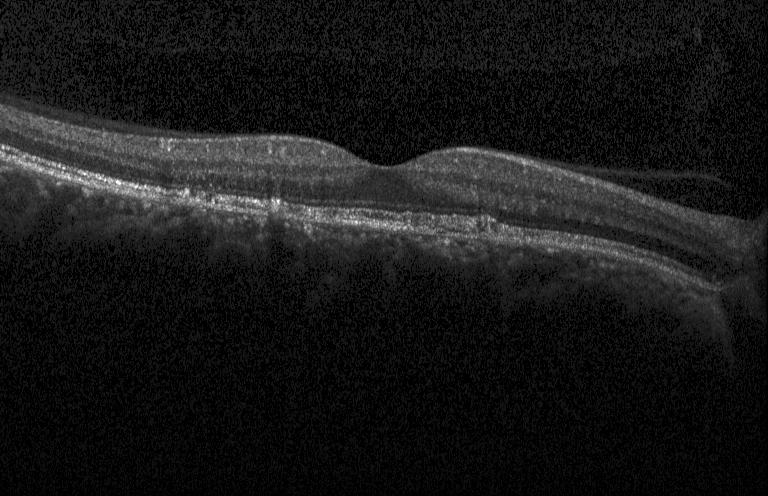 Retinal OCT B-scan · SD-OCT · instrument: Heidelberg Spectralis. Finding: drusen.